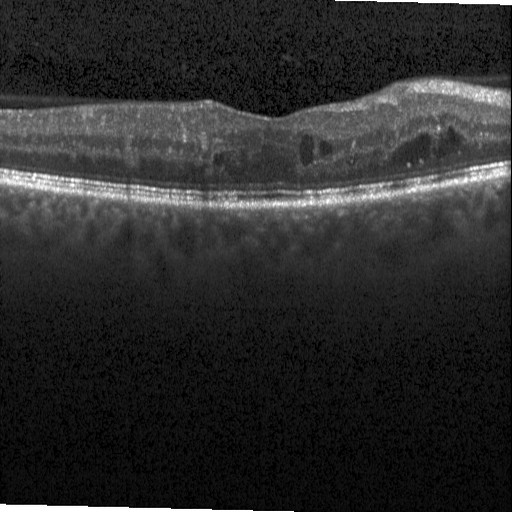
Dx: DME.